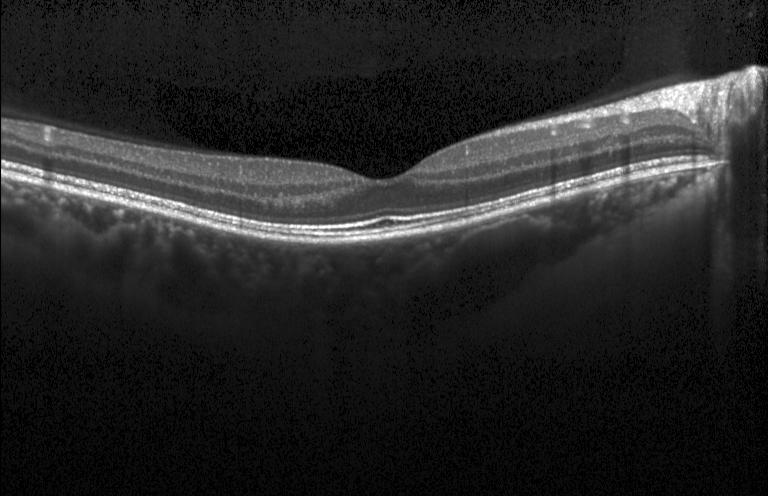
OCT scan showing no CNV, no DME, and no drusen.